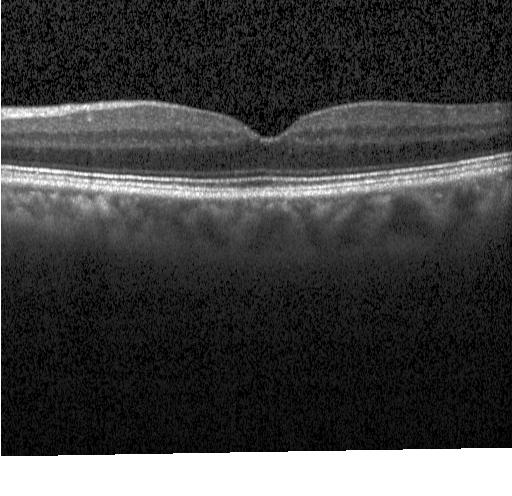

Retinal OCT cross-section showing neither choroidal neovascularization, diabetic macular edema, nor drusen.